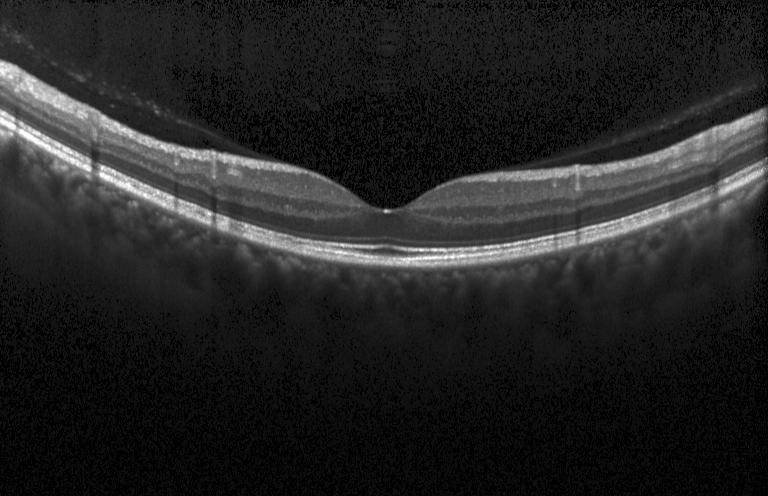
Heidelberg Spectralis OCT system · fovea-centered · OCT B-scan · spectral-domain optical coherence tomography.
Assessment: no CNV, no DME, and no drusen.